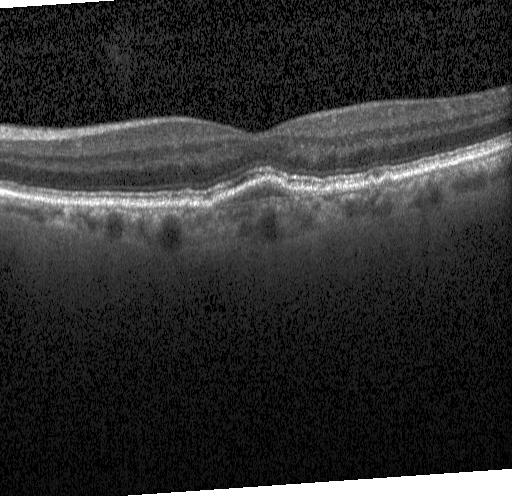

Choroidal neovascularization (CNV).